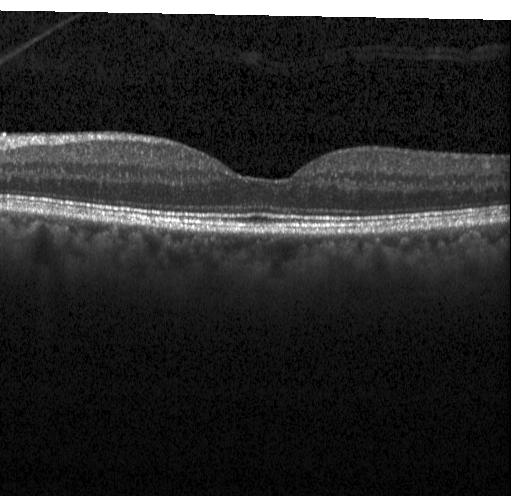

The scan shows no choroidal neovascularization, diabetic macular edema, or drusen.